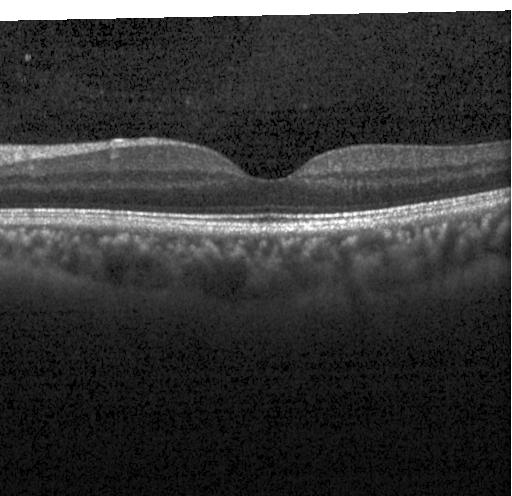
Fovea-centered; retinal OCT cross-section. OCT finding: no choroidal neovascularization, diabetic macular edema, or drusen.